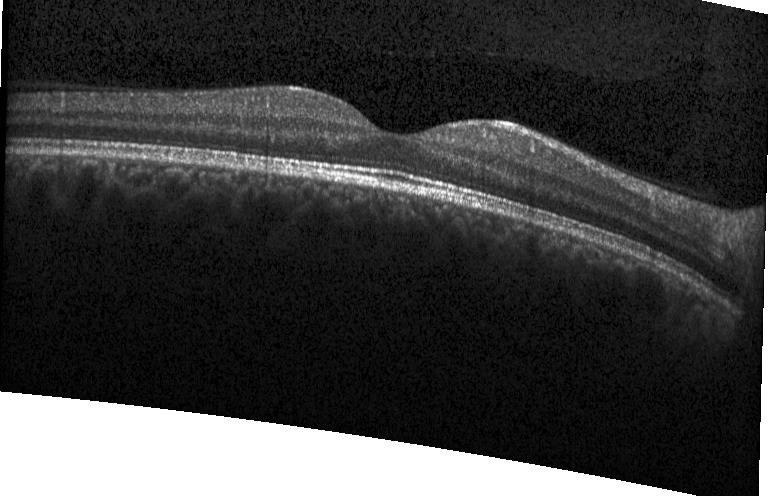
Optical coherence tomography B-scan
This B-scan demonstrates no evidence of CNV, DME, or drusen.